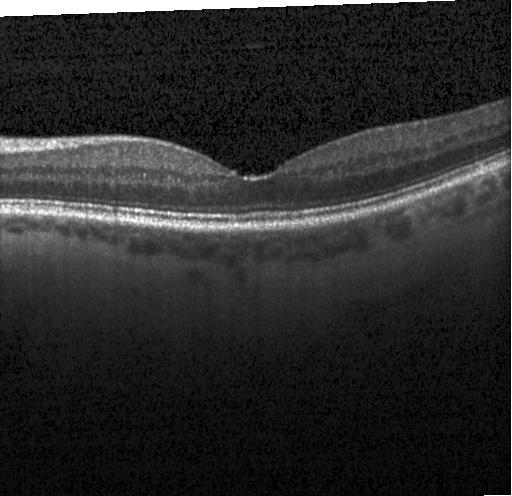

Retinal OCT B-scan. Spectral-domain OCT. Through the macula. Acquired on a Heidelberg Spectralis.
Dx: no evidence of choroidal neovascularization, diabetic macular edema, or drusen.